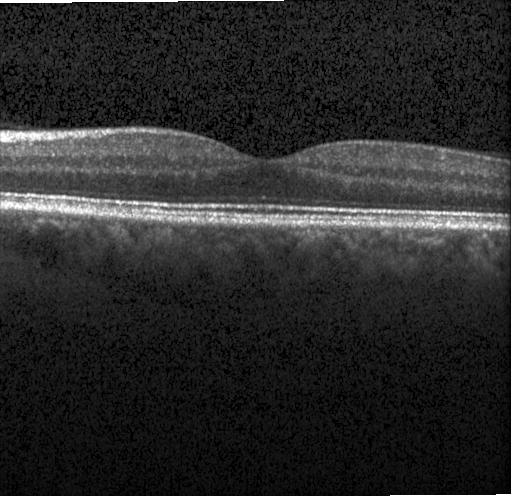 Impression: no choroidal neovascularization, no diabetic macular edema, and no drusen.